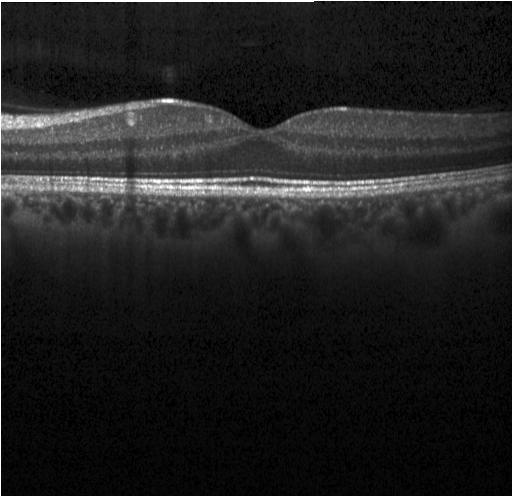

OCT finding: no choroidal neovascularization, diabetic macular edema, or drusen.